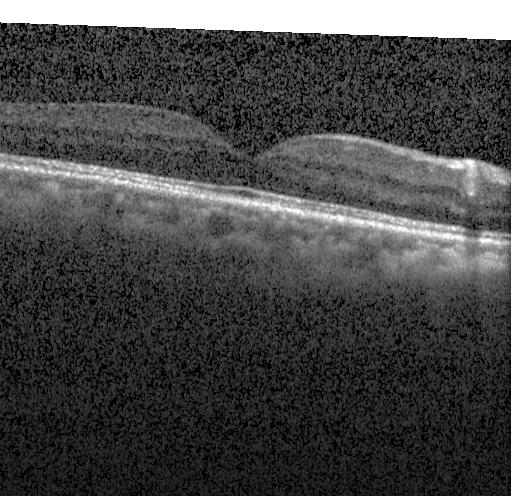

Impression: no choroidal neovascularization, diabetic macular edema, or drusen.